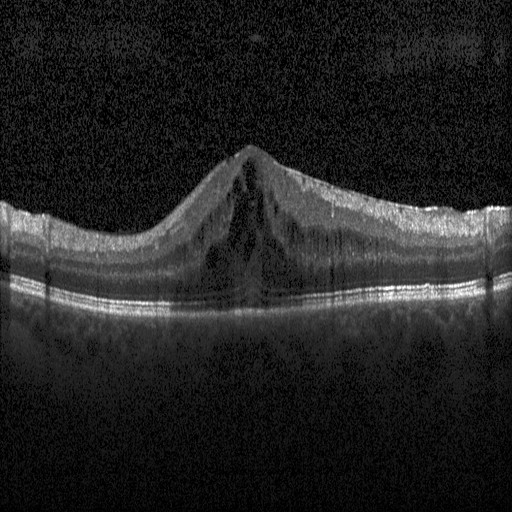

Spectral-domain OCT B-scan: DME.